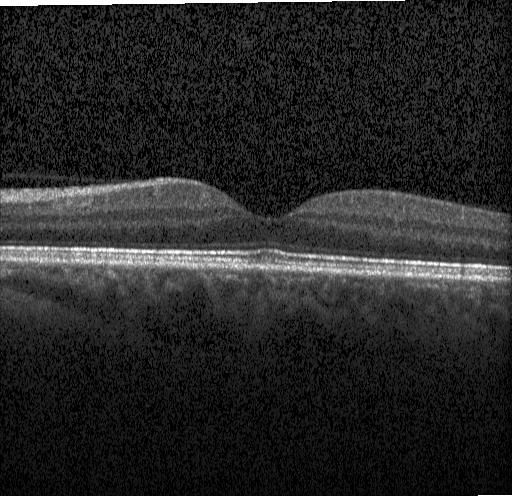

Instrument: Heidelberg Spectralis · retinal OCT cross-section · through the macula · SD-OCT.
The scan shows neither CNV, DME, nor drusen.